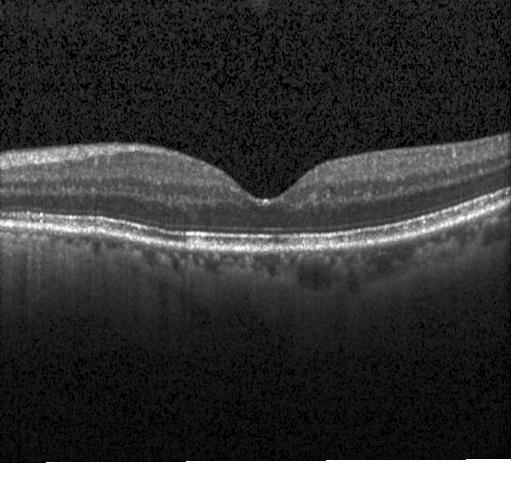 Macular OCT: no choroidal neovascularization, no diabetic macular edema, and no drusen.